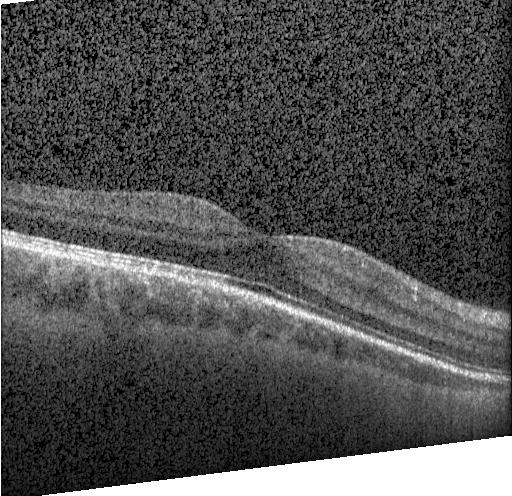 Heidelberg Spectralis, horizontal scan through the fovea, optical coherence tomography scan.
The scan shows no choroidal neovascularization, no diabetic macular edema, and no drusen.